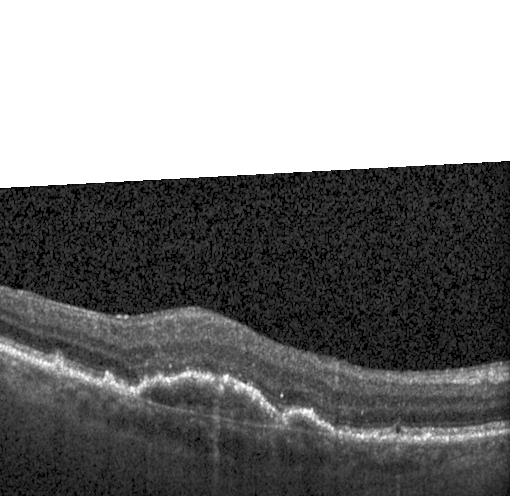
Optical coherence tomography scan. Diagnosis: a choroidal neovascular membrane.